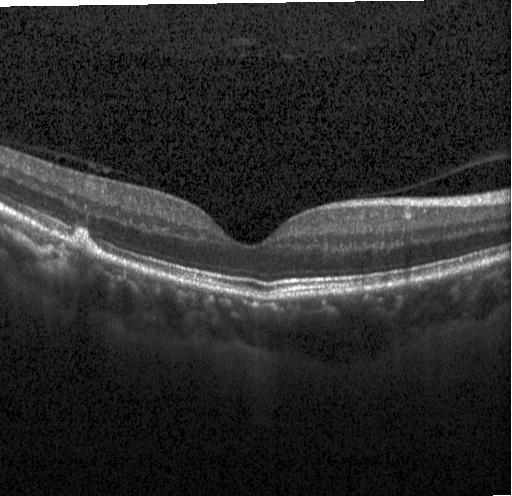 Impression: multiple drusen.